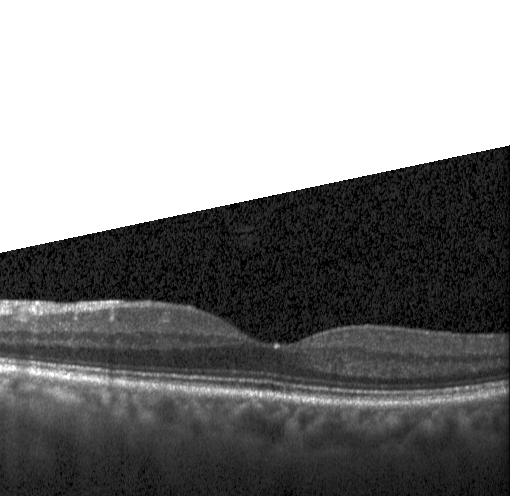

Acquired on a Heidelberg Spectralis · spectral-domain optical coherence tomography · retinal OCT B-scan · through the macula.
Diagnosis: neither choroidal neovascularization, diabetic macular edema, nor drusen.